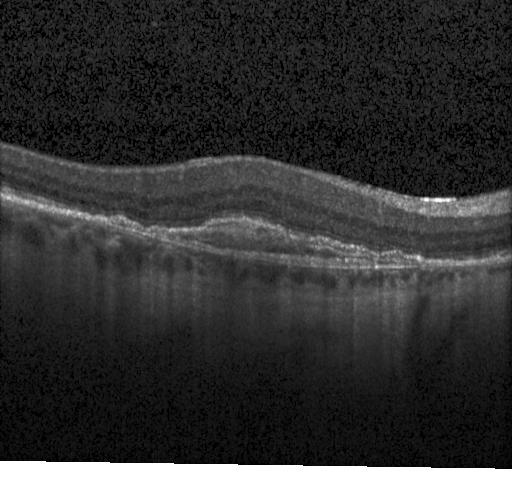

Optical coherence tomography scan — Impression: a choroidal neovascular membrane.